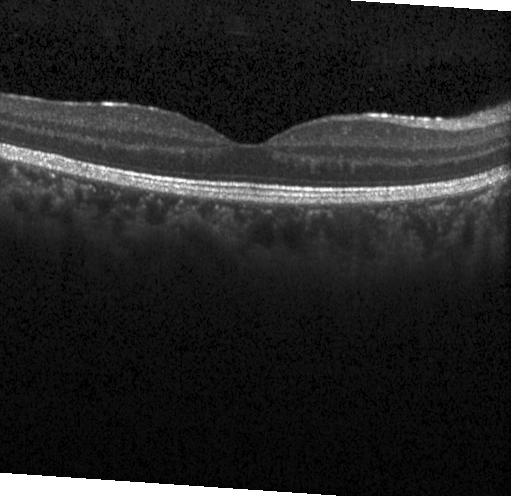

Macular scan; spectral-domain OCT; OCT B-scan. Macular OCT: neither choroidal neovascularization, diabetic macular edema, nor drusen.